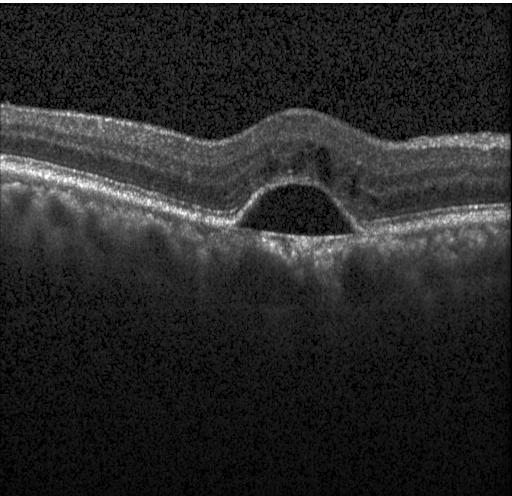 Heidelberg Spectralis. Spectral-domain optical coherence tomography. Fovea-centered. OCT B-scan. This B-scan demonstrates a choroidal neovascular membrane.